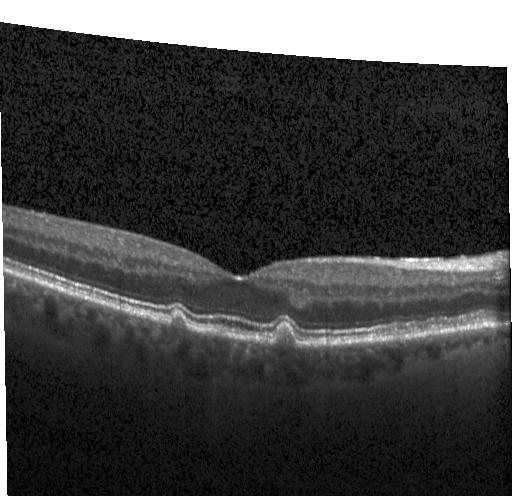
Finding: drusen.